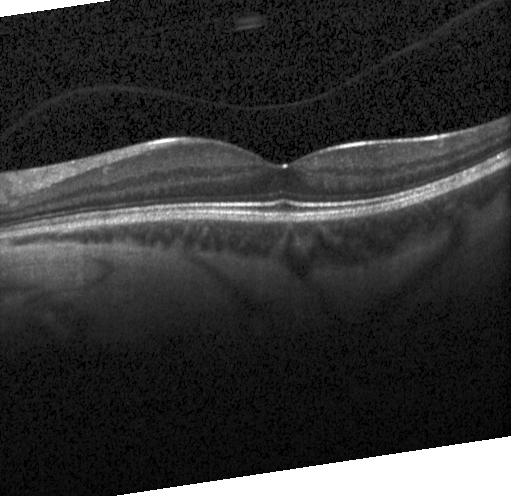

Impression: no CNV, DME, or drusen.